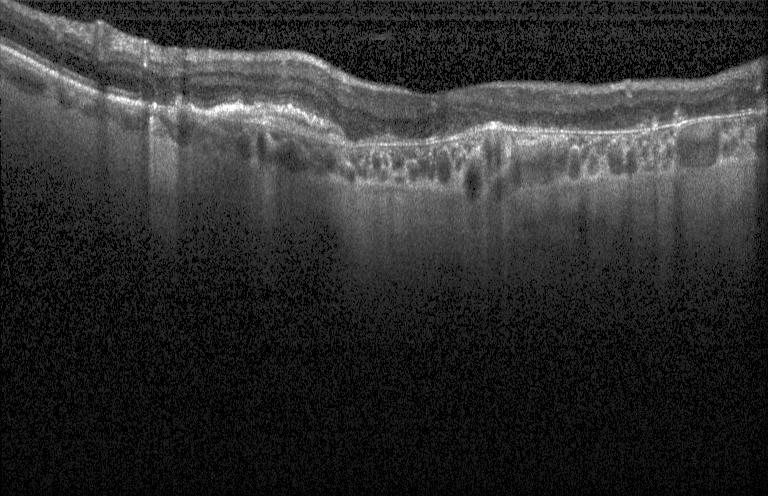

Optical coherence tomography scan; fovea-centered.
Finding: CNV.